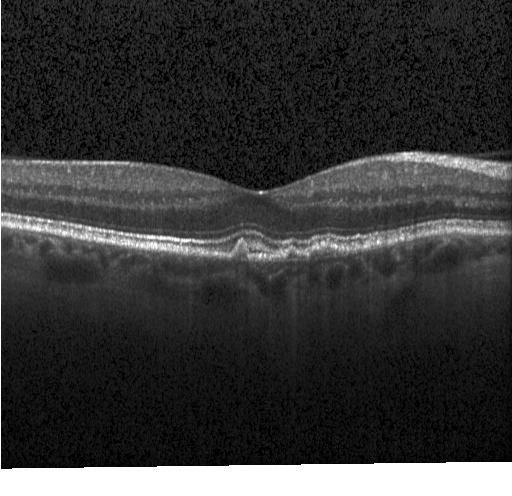

Spectral-domain optical coherence tomography; OCT B-scan; centered on the fovea
This B-scan demonstrates drusen.